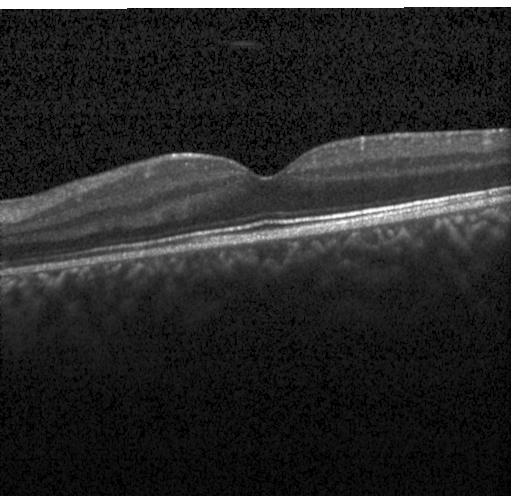

Macular OCT: neither CNV, DME, nor drusen.